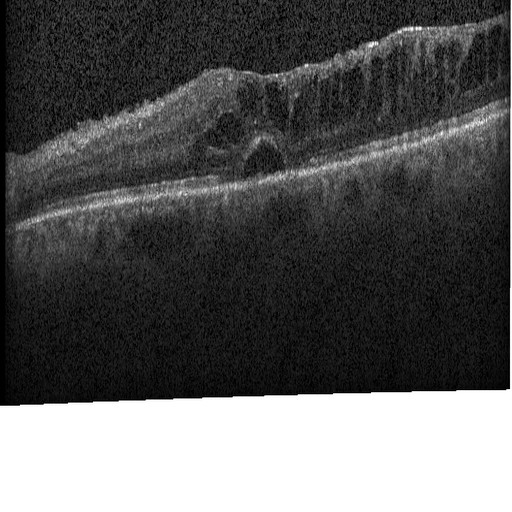
Acquired on a Heidelberg Spectralis, optical coherence tomography scan, spectral-domain optical coherence tomography — Diagnosis: diabetic macular edema (DME).